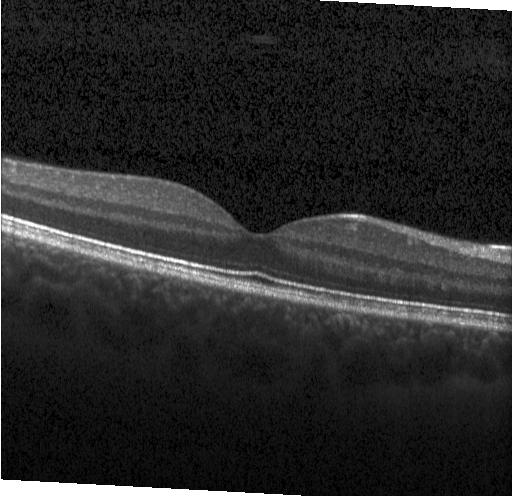

Spectral-domain OCT, instrument: Heidelberg Spectralis, OCT B-scan, centered on the fovea.
Finding: no evidence of choroidal neovascularization, diabetic macular edema, or drusen.